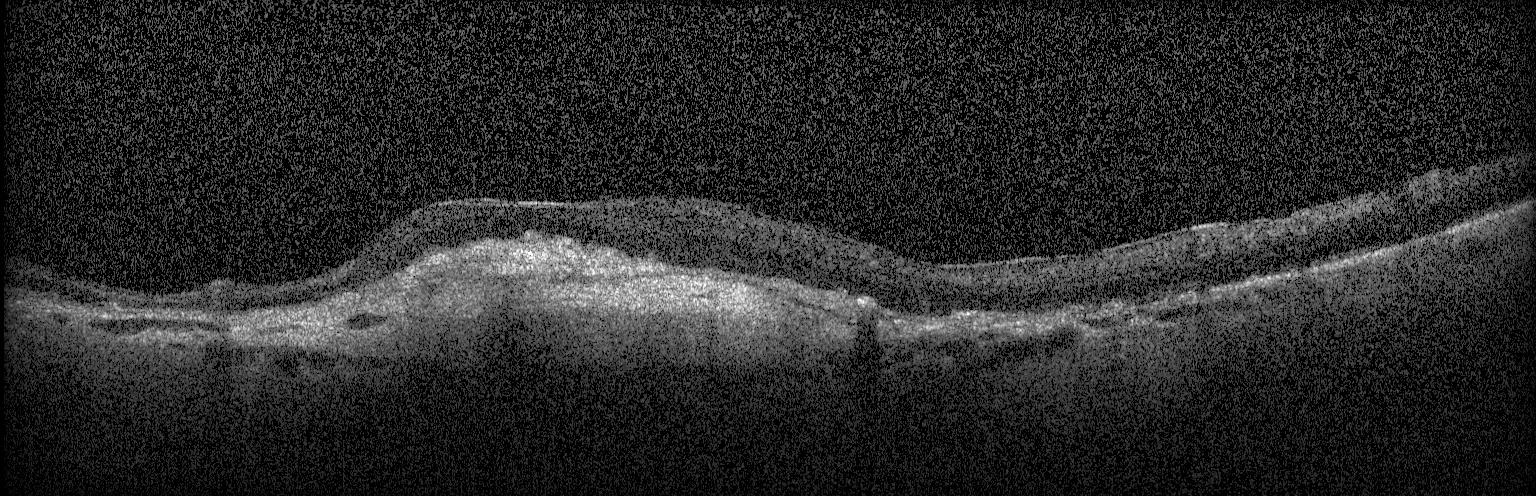
Dx: a choroidal neovascular membrane.